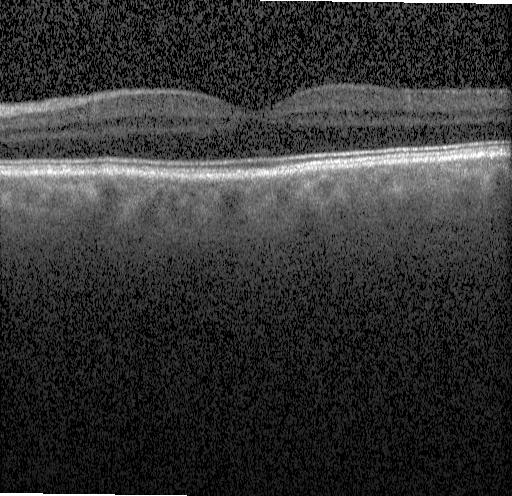

OCT finding: neither choroidal neovascularization, diabetic macular edema, nor drusen.